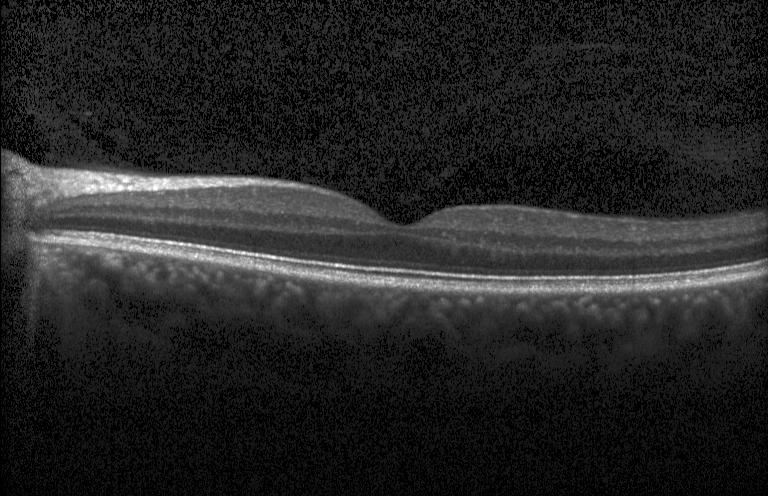

Retinal OCT cross-section.
Finding: no evidence of choroidal neovascularization, diabetic macular edema, or drusen.